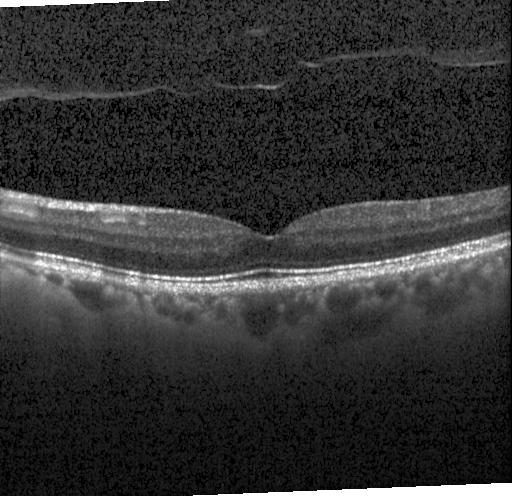 Retinal OCT B-scan; centered on the fovea.
The scan shows neither choroidal neovascularization, diabetic macular edema, nor drusen.